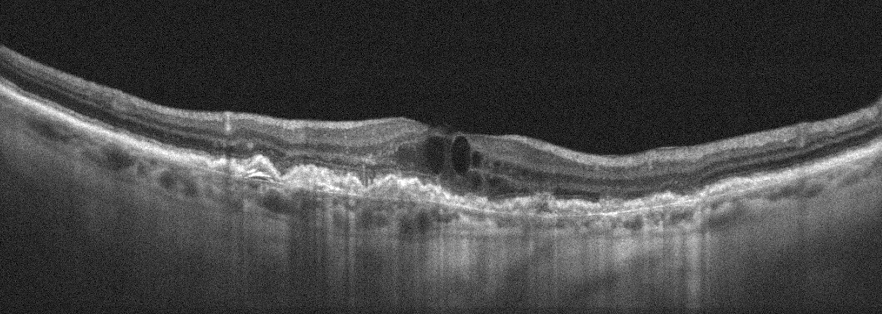

Optical coherence tomography scan, fovea-centered, instrument: Optovue Avanti RTVue XR, OD — Assessment: age-related macular degeneration (AMD).